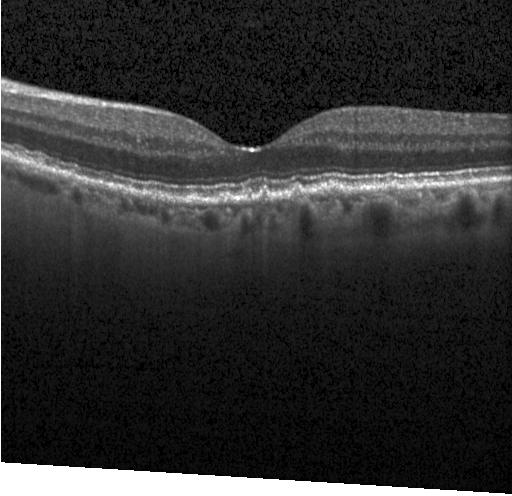

Horizontal scan through the fovea. Optical coherence tomography scan. Spectral-domain optical coherence tomography. Instrument: Heidelberg Spectralis
Finding: multiple drusen.